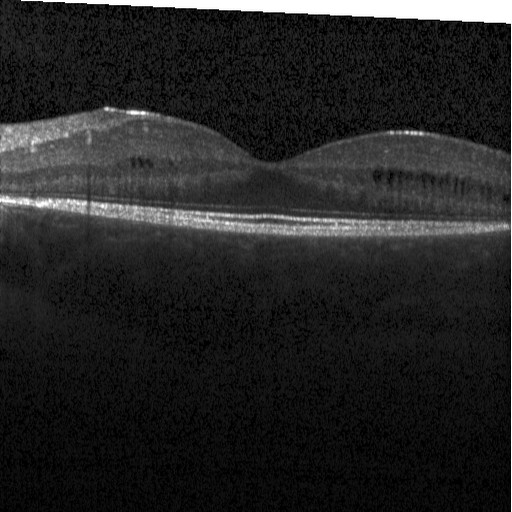 Centered on the fovea · Heidelberg Spectralis · OCT line scan. Assessment: diabetic macular edema (DME).